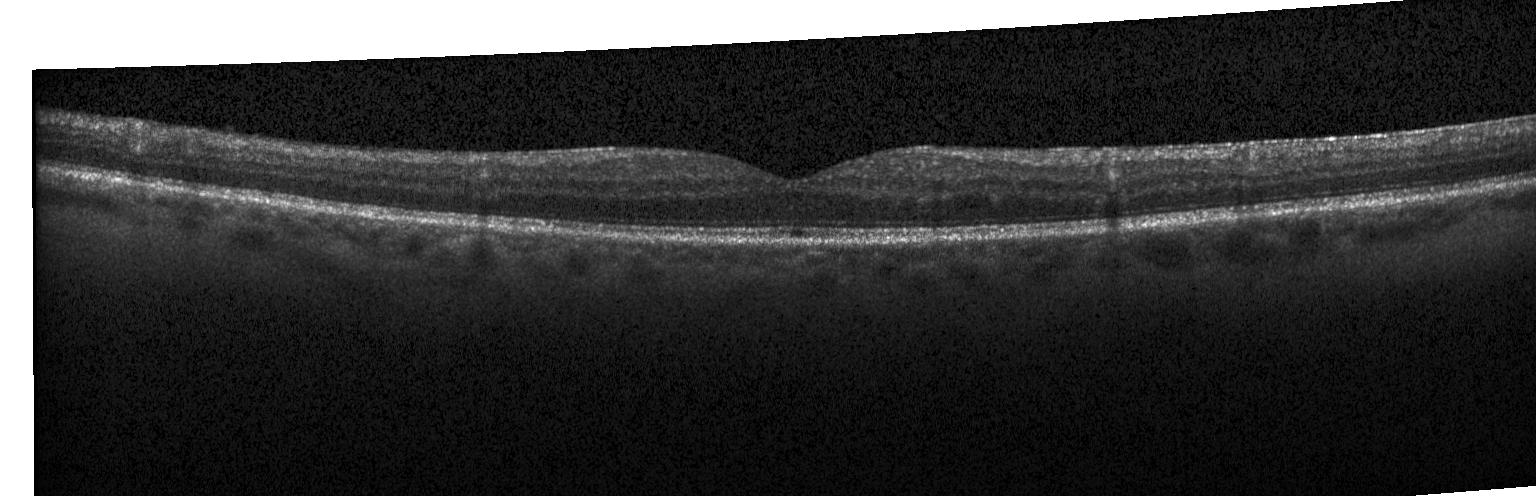

Retinal OCT cross-section, through the macula — The scan shows neither choroidal neovascularization, diabetic macular edema, nor drusen.